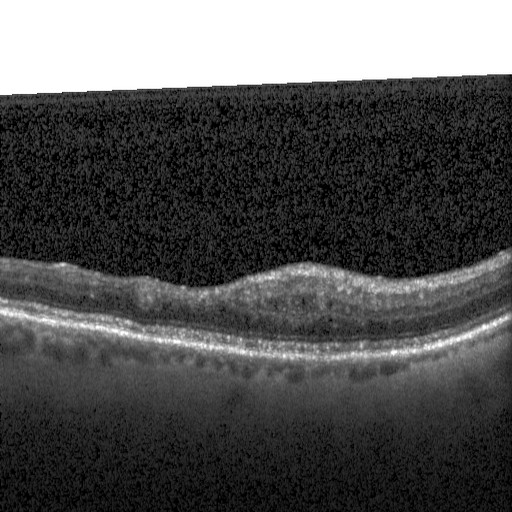 Horizontal scan through the fovea. Retinal OCT cross-section. Spectral-domain OCT.
The scan shows DME.